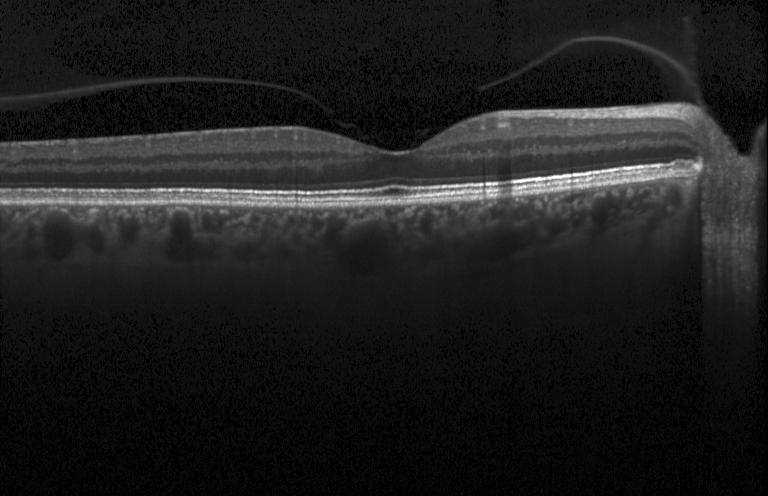 Macular OCT: neither choroidal neovascularization, diabetic macular edema, nor drusen.